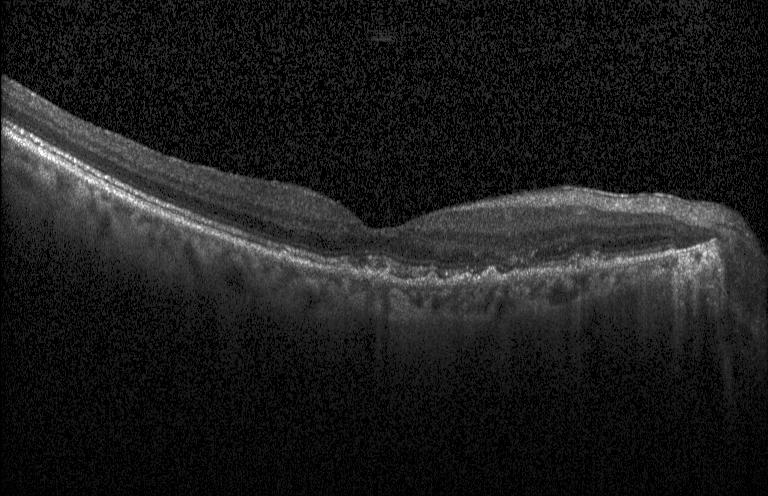
Optical coherence tomography scan. Assessment: a choroidal neovascular membrane.